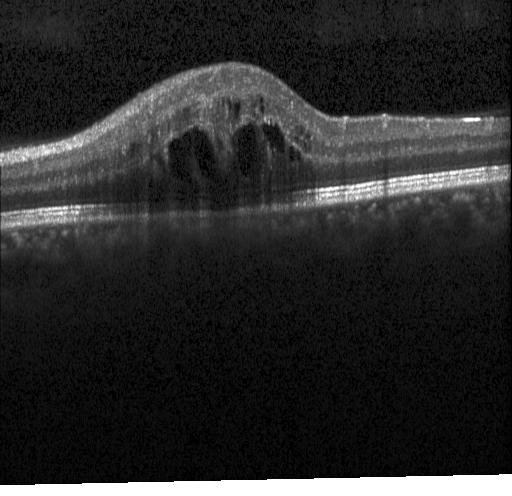

OCT line scan. Finding: diabetic macular edema (DME).